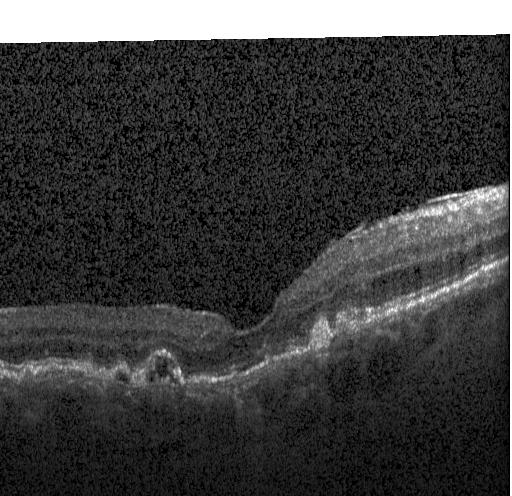 Optical coherence tomography B-scan; instrument: Heidelberg Spectralis; spectral-domain optical coherence tomography; macular scan — Diagnosis: a choroidal neovascular membrane.